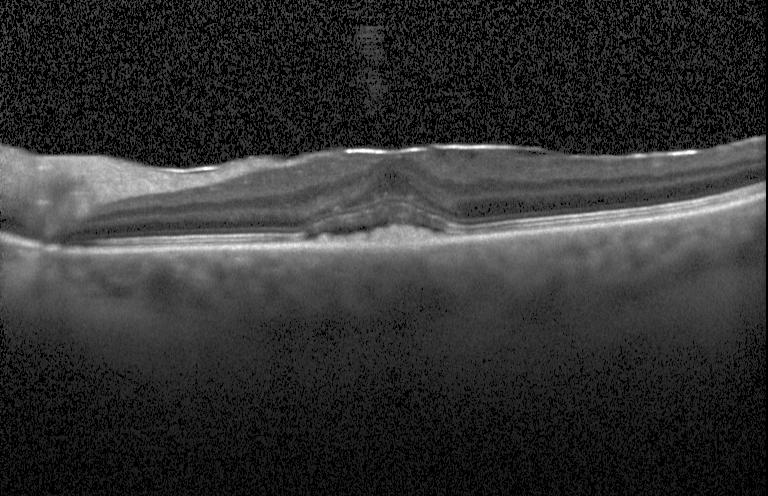

Retinal OCT B-scan, acquired on a Heidelberg Spectralis — Diagnosis: choroidal neovascularization.